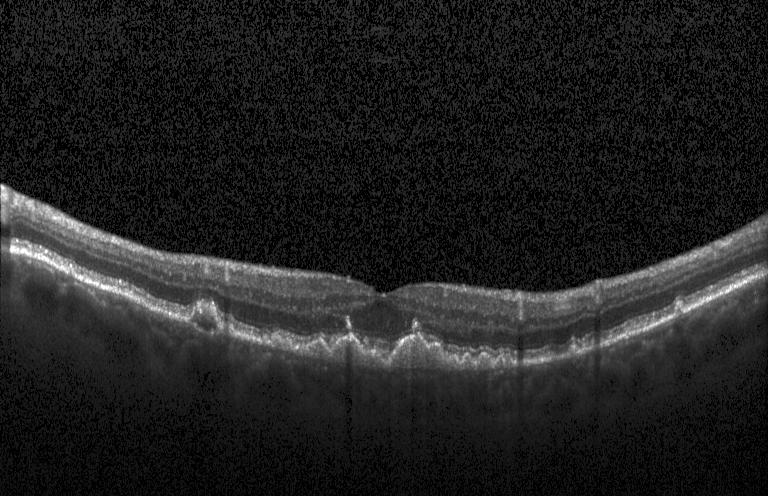

Instrument: Heidelberg Spectralis. Through the macula. Retinal OCT cross-section. Impression: sub-RPE drusenoid deposits.